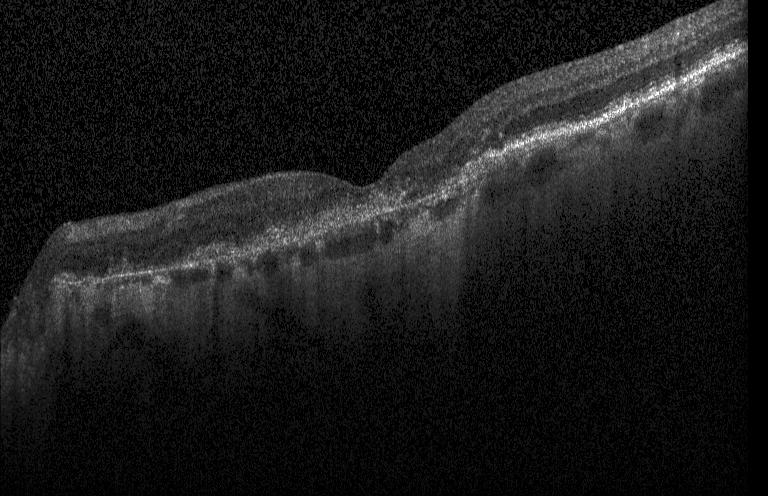

OCT B-scan. SD-OCT — Diagnosis: a choroidal neovascular membrane.